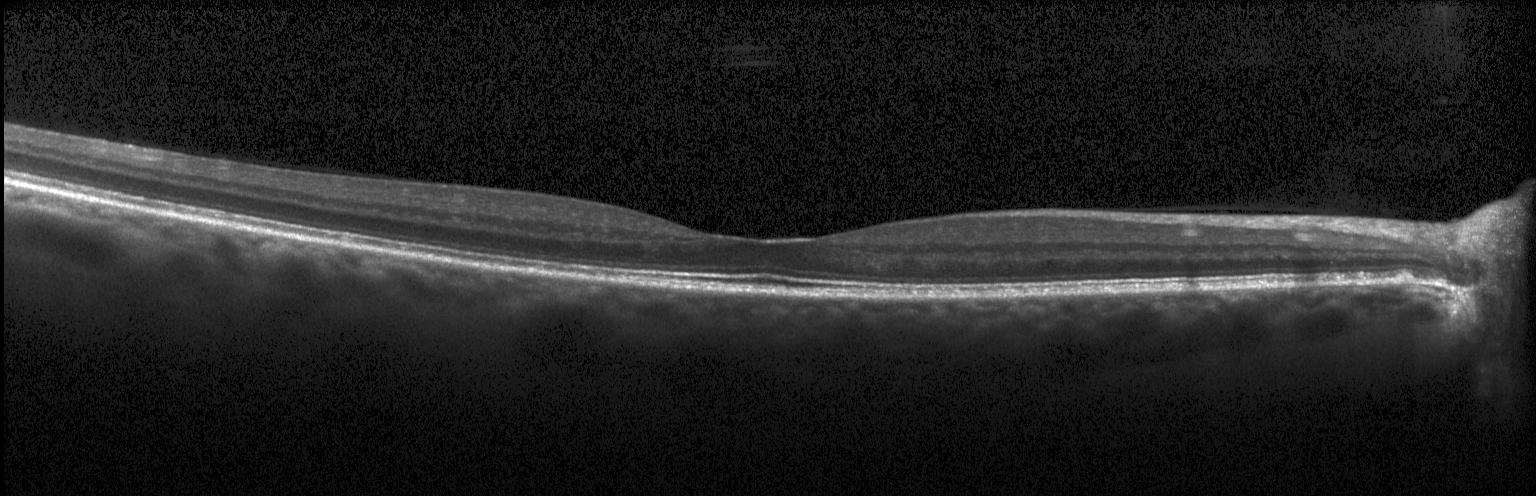

Optical coherence tomography B-scan
Diagnosis: no CNV, no DME, and no drusen.